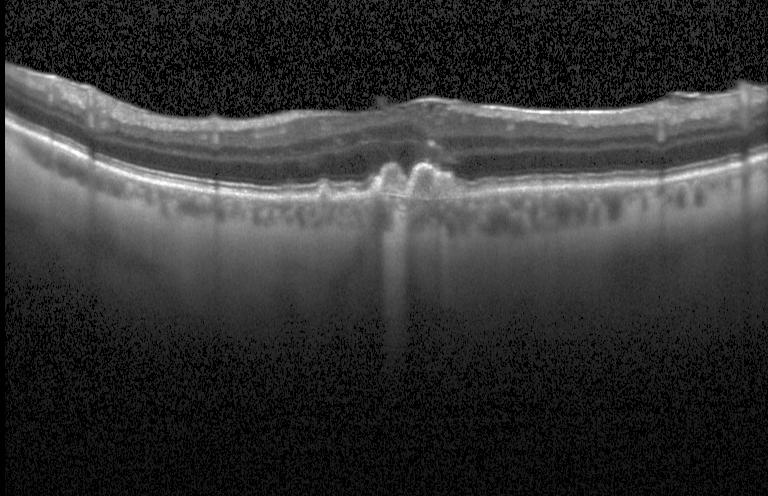
Optical coherence tomography scan.
Diagnosis: sub-RPE drusenoid deposits.